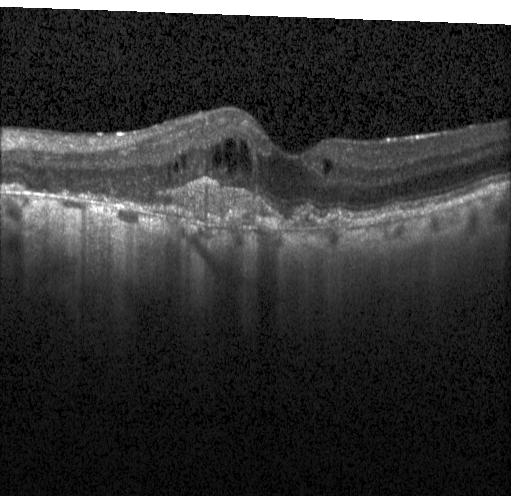

Impression: choroidal neovascularization (CNV).